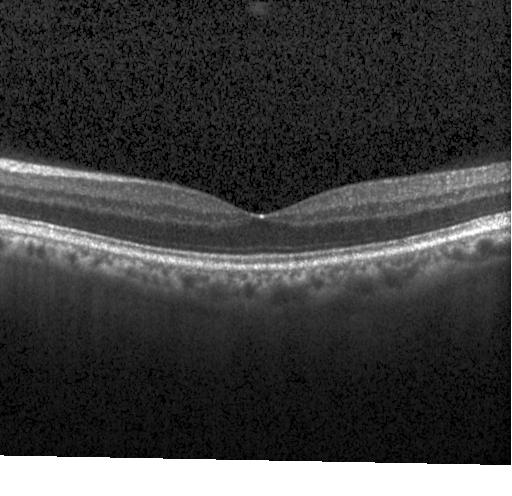

OCT finding: no CNV, no DME, and no drusen.